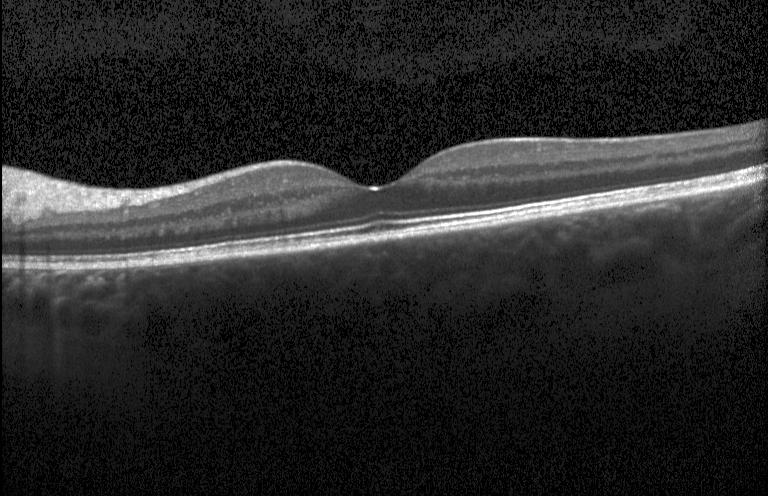 Optical coherence tomography B-scan — Finding: neither CNV, DME, nor drusen.